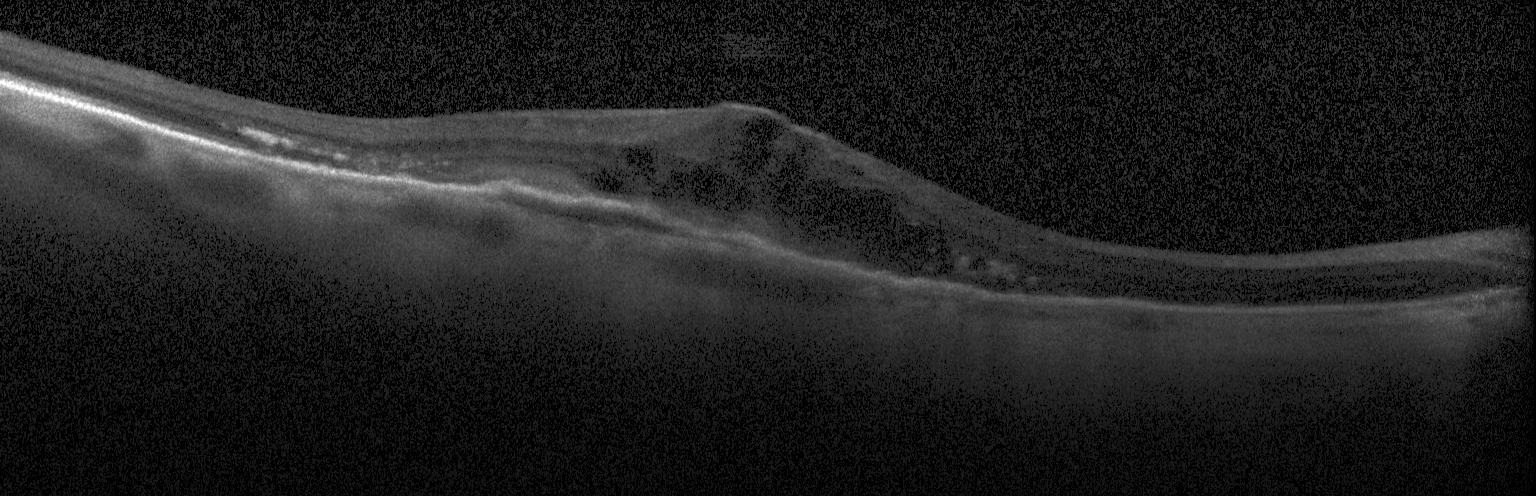 Spectral-domain optical coherence tomography. Optical coherence tomography B-scan. Heidelberg Spectralis OCT system. Centered on the fovea
Impression: CNV.